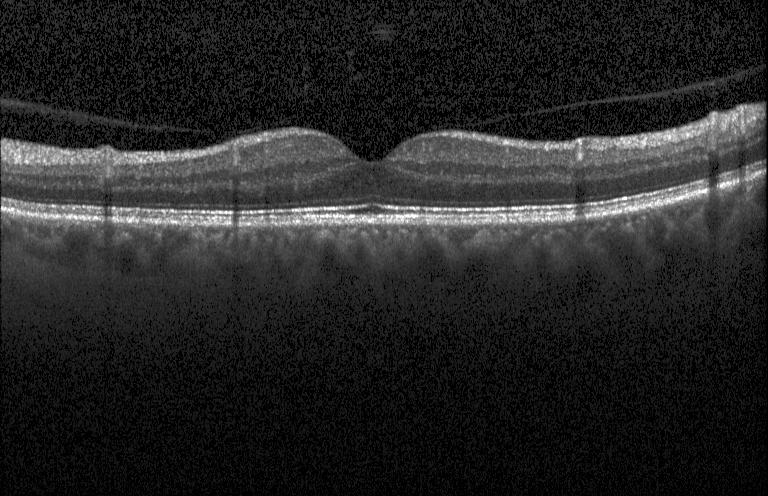
Spectral-domain optical coherence tomography. Optical coherence tomography B-scan — Dx: no choroidal neovascularization, no diabetic macular edema, and no drusen.